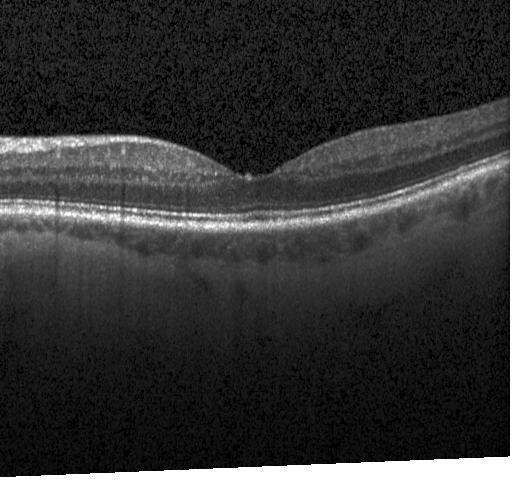
This B-scan demonstrates no evidence of choroidal neovascularization, diabetic macular edema, or drusen.